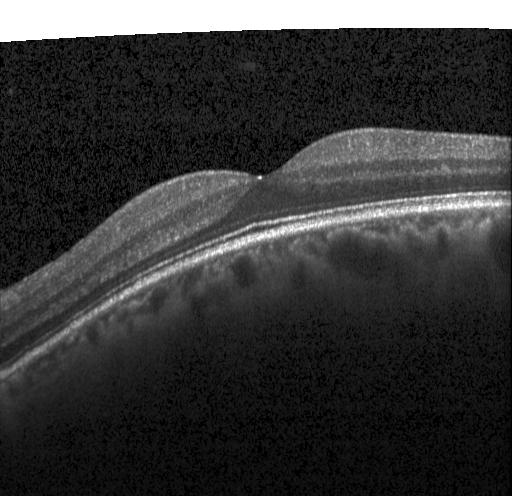 Retinal OCT cross-section, acquired on a Heidelberg Spectralis.
Finding: neither choroidal neovascularization, diabetic macular edema, nor drusen.